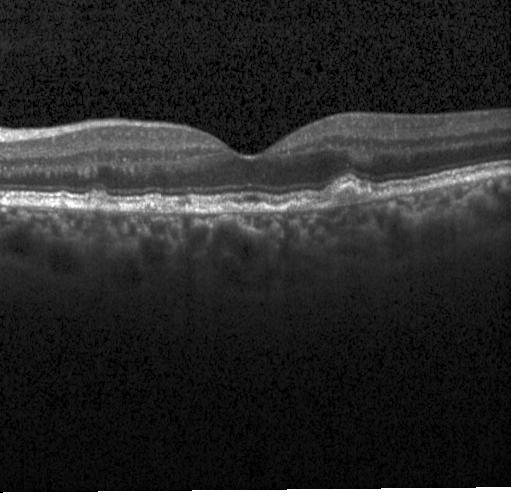
Optical coherence tomography B-scan, Heidelberg Spectralis.
Multiple drusen.